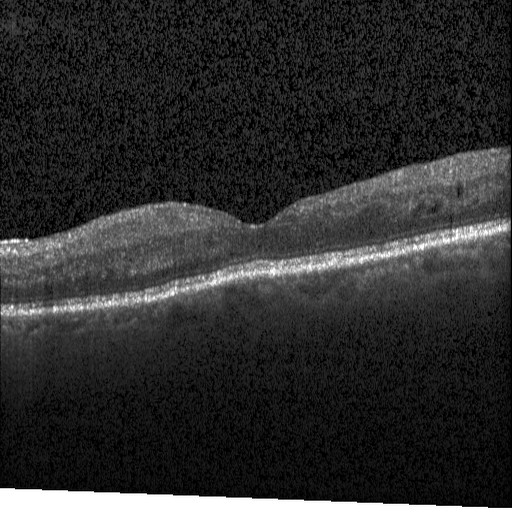

Macular OCT demonstrating diabetic macular edema (DME).